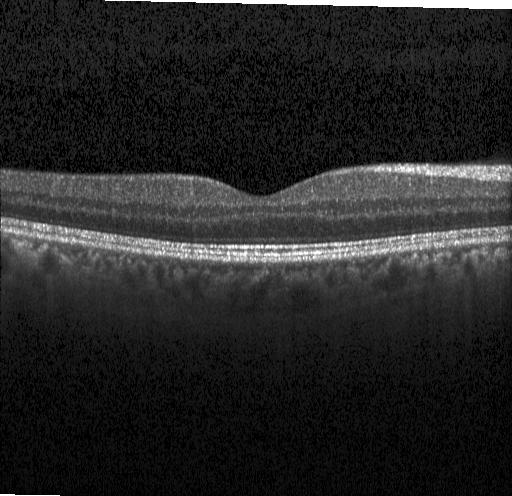
SD-OCT. OCT line scan. Centered on the fovea. Heidelberg Spectralis.
Impression: no evidence of choroidal neovascularization, diabetic macular edema, or drusen.